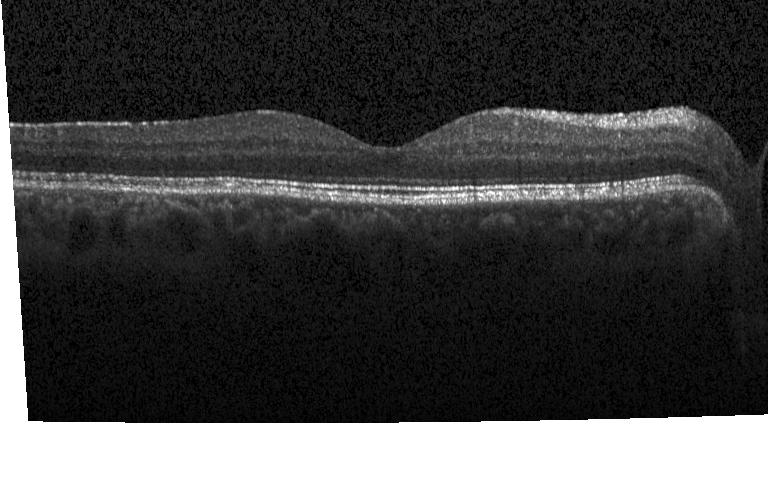 Horizontal scan through the fovea. Spectral-domain optical coherence tomography. OCT line scan. Finding: no evidence of choroidal neovascularization, diabetic macular edema, or drusen.